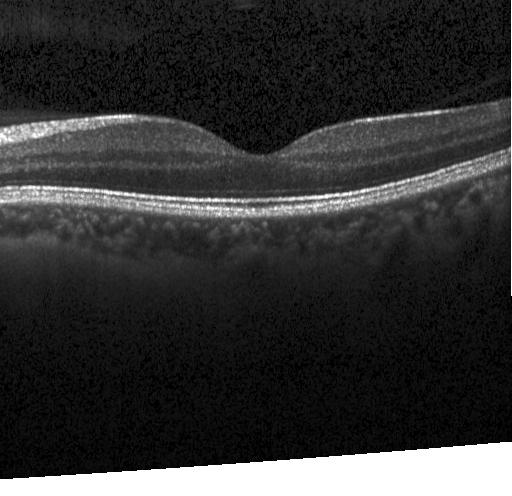 Heidelberg Spectralis OCT system. Retinal OCT cross-section. Horizontal scan through the fovea — The scan shows no evidence of CNV, DME, or drusen.